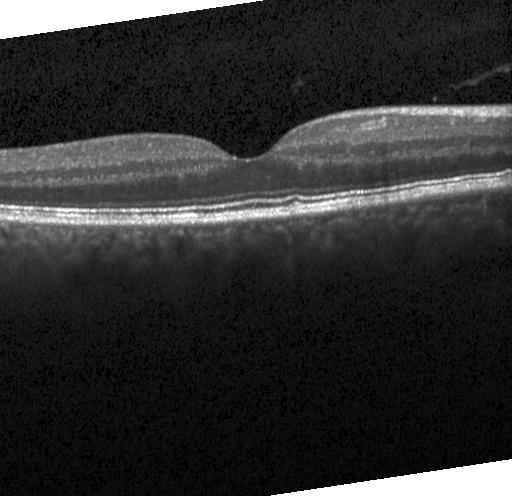
Retinal OCT cross-section showing no evidence of choroidal neovascularization, diabetic macular edema, or drusen.